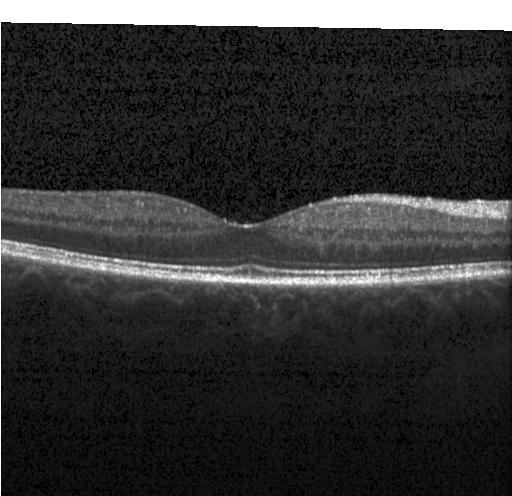 Acquired on a Heidelberg Spectralis · optical coherence tomography B-scan — No choroidal neovascularization, diabetic macular edema, or drusen.